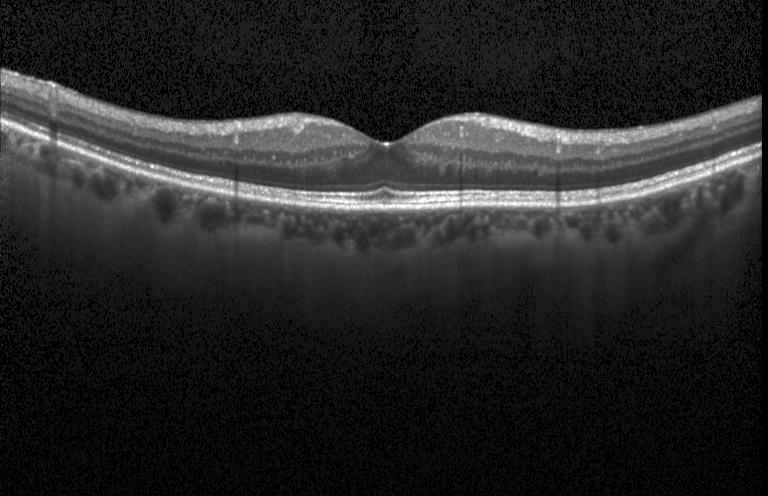
Centered on the fovea · optical coherence tomography B-scan · Heidelberg Spectralis
Assessment: neither choroidal neovascularization, diabetic macular edema, nor drusen.